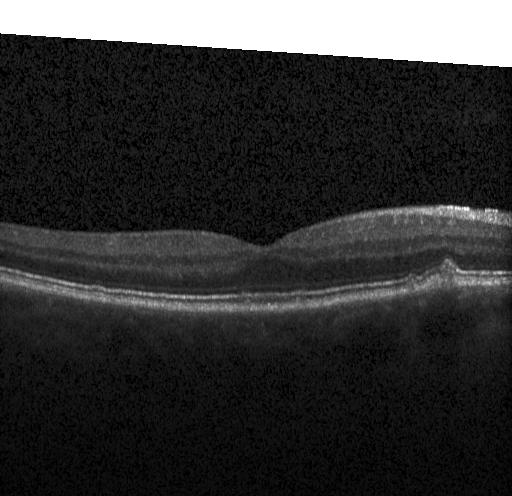
OCT finding: drusen.